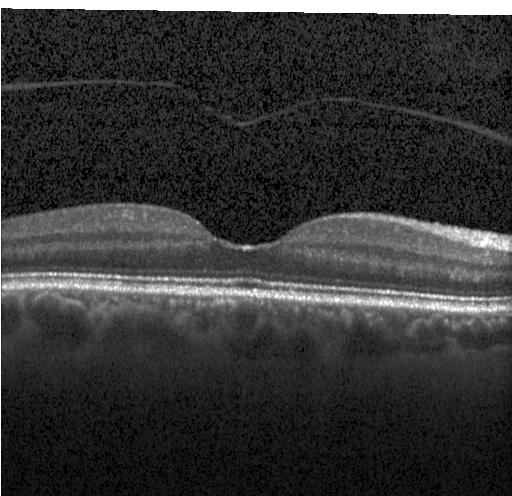 OCT B-scan.
OCT finding: no choroidal neovascularization, diabetic macular edema, or drusen.